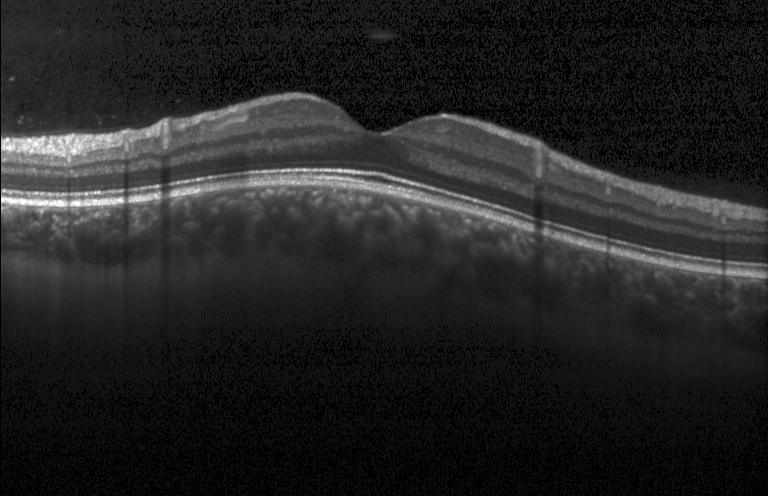
OCT line scan; instrument: Heidelberg Spectralis; fovea-centered; spectral-domain OCT.
No choroidal neovascularization, diabetic macular edema, or drusen.